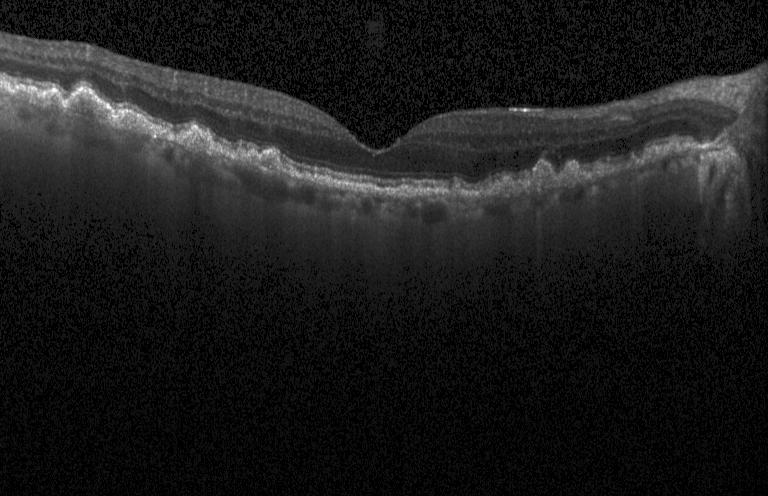
Optical coherence tomography scan. Impression: drusen.